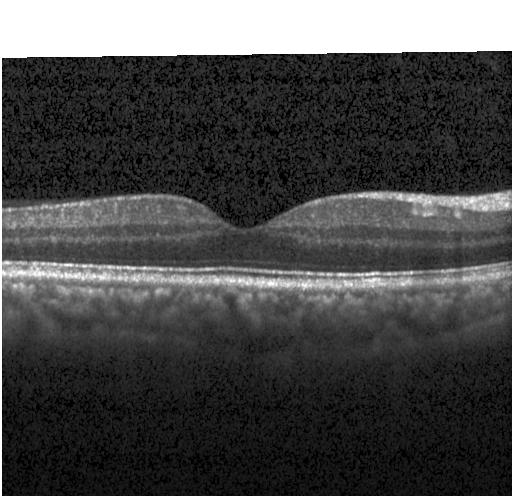

Finding: no evidence of choroidal neovascularization, diabetic macular edema, or drusen.